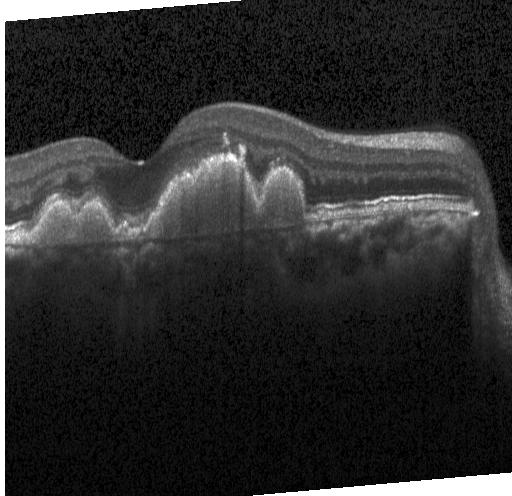
Retinal OCT B-scan. Through the macula
This B-scan demonstrates sub-RPE drusenoid deposits.